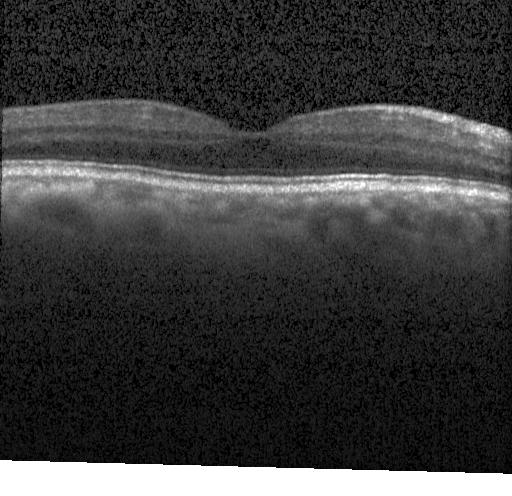 Impression: no CNV, DME, or drusen.